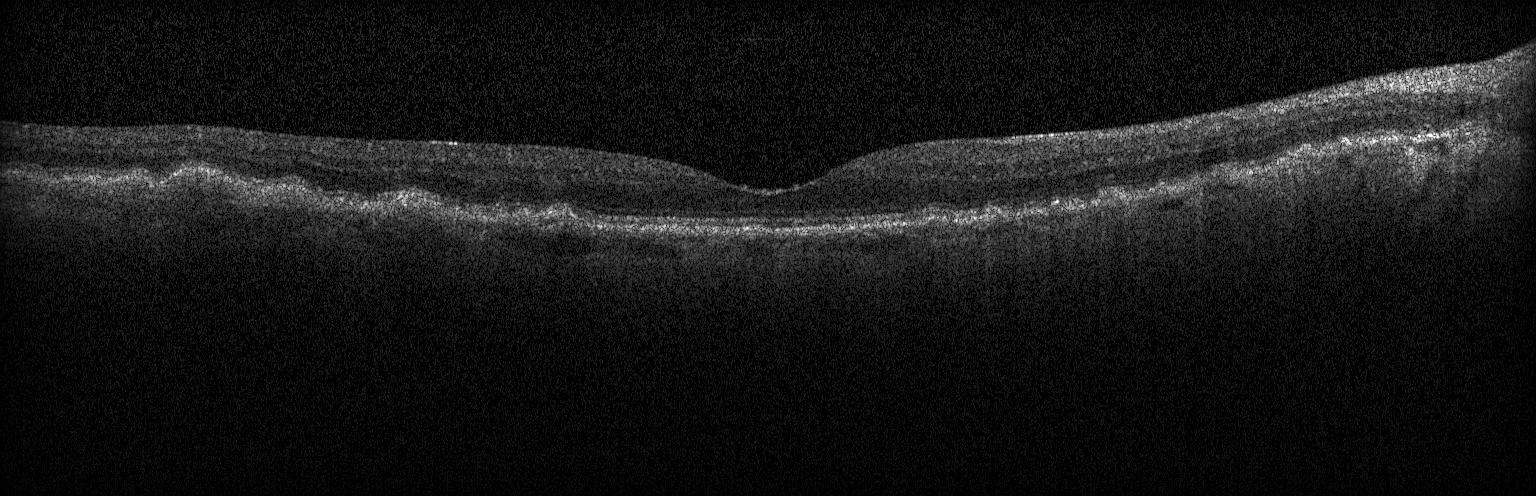
Finding: multiple drusen.